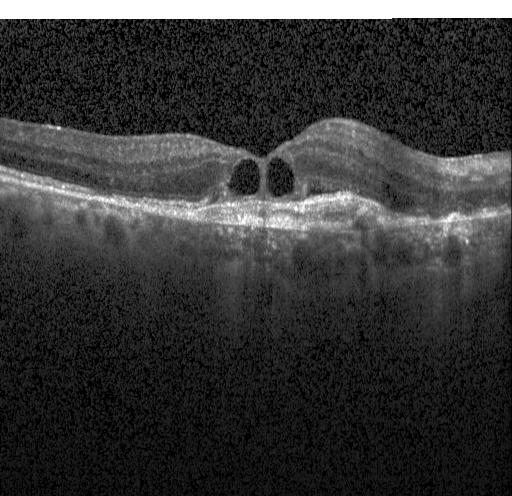

Finding: a choroidal neovascular membrane.